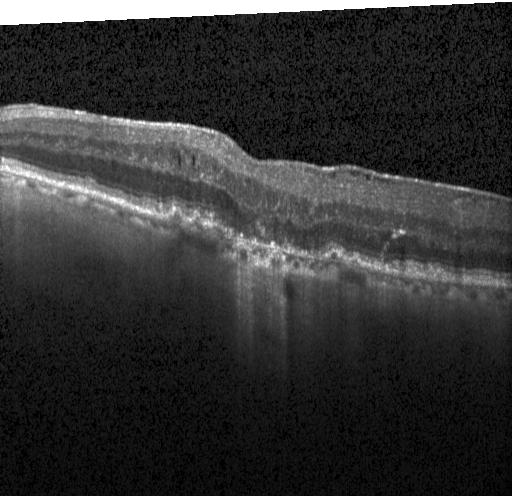 Optical coherence tomography scan
A choroidal neovascular membrane.